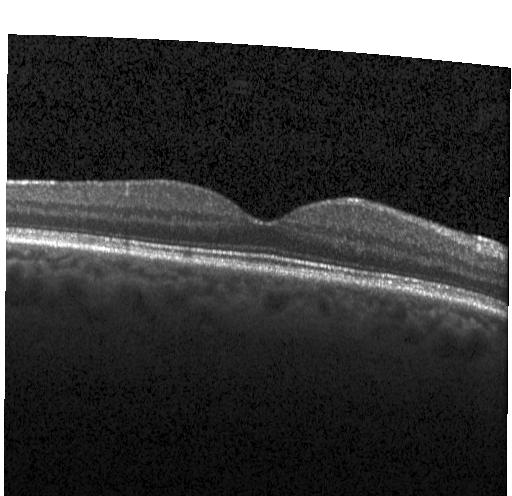 Spectral-domain optical coherence tomography, centered on the fovea, OCT line scan, acquired on a Heidelberg Spectralis
This B-scan demonstrates no choroidal neovascularization, no diabetic macular edema, and no drusen.